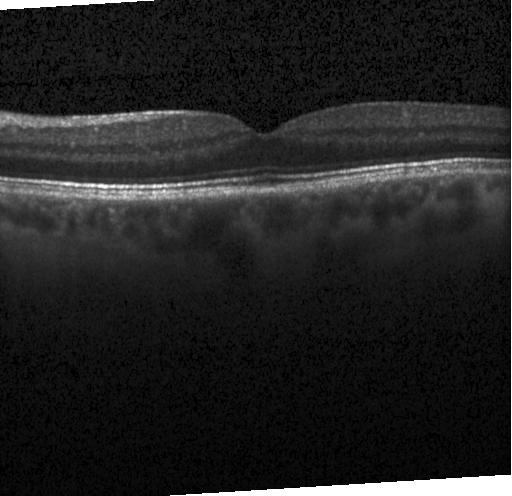 Spectral-domain OCT, acquired on a Heidelberg Spectralis, optical coherence tomography B-scan — Finding: no choroidal neovascularization, diabetic macular edema, or drusen.